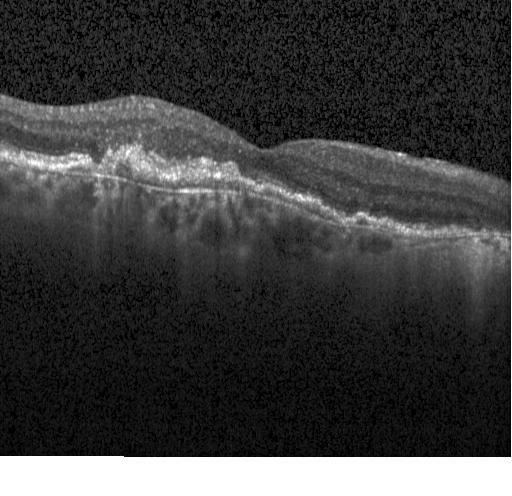

OCT finding: choroidal neovascularization (CNV).